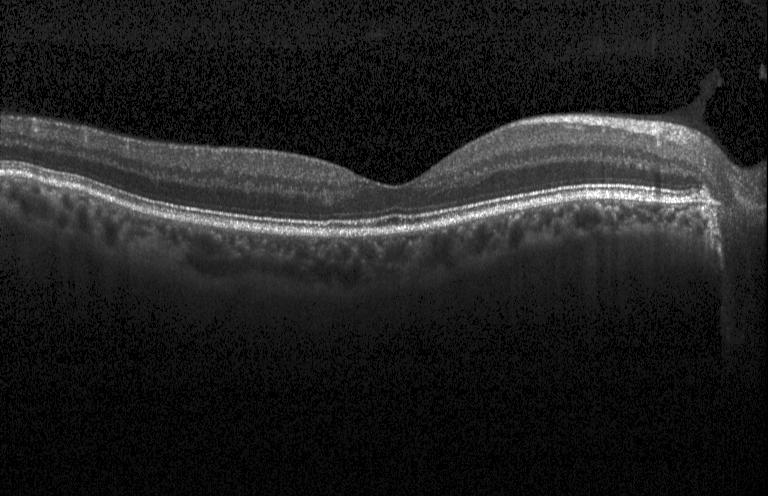
Optical coherence tomography B-scan; fovea-centered. This B-scan demonstrates no choroidal neovascularization, no diabetic macular edema, and no drusen.